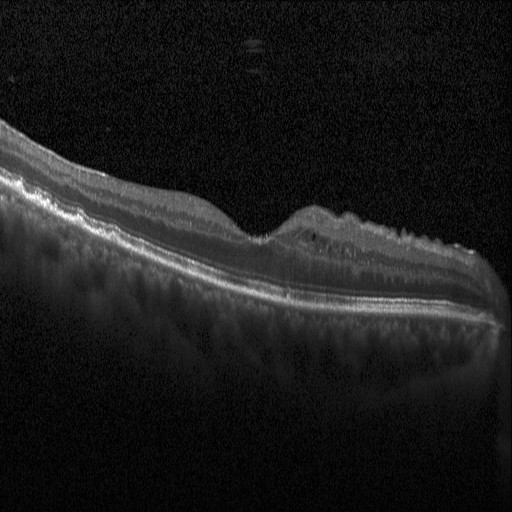

Retinal OCT cross-section showing diabetic macular edema.